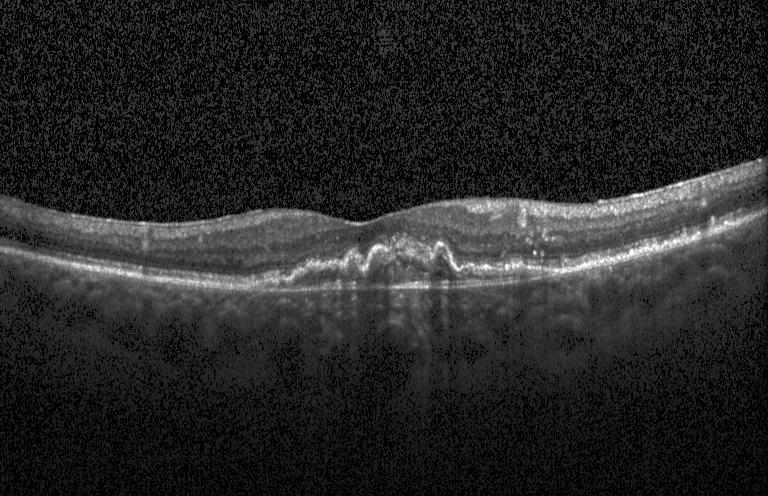 OCT B-scan, Heidelberg Spectralis, spectral-domain optical coherence tomography
This B-scan demonstrates a choroidal neovascular membrane.